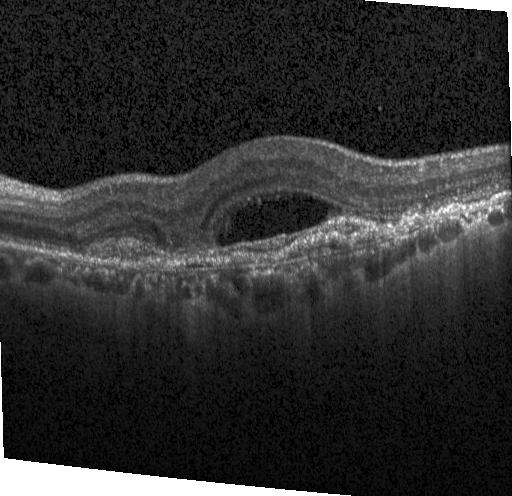

Optical coherence tomography scan · macular scan · instrument: Heidelberg Spectralis — Finding: a choroidal neovascular membrane.